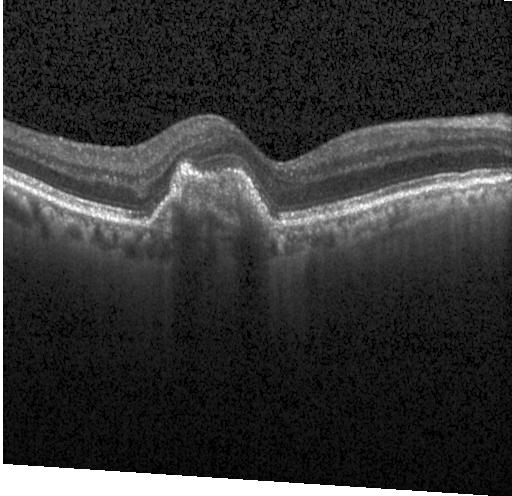

Spectral-domain optical coherence tomography. Optical coherence tomography B-scan
Finding: choroidal neovascularization.